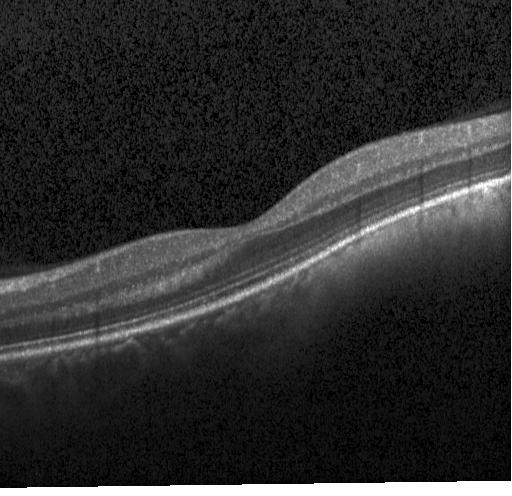 Diagnosis: no choroidal neovascularization, no diabetic macular edema, and no drusen.